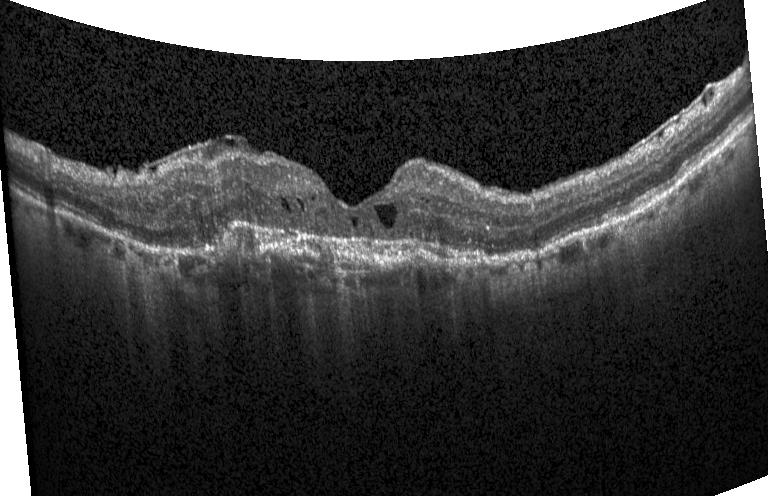

Heidelberg Spectralis OCT system. Optical coherence tomography B-scan. Diagnosis: a choroidal neovascular membrane.